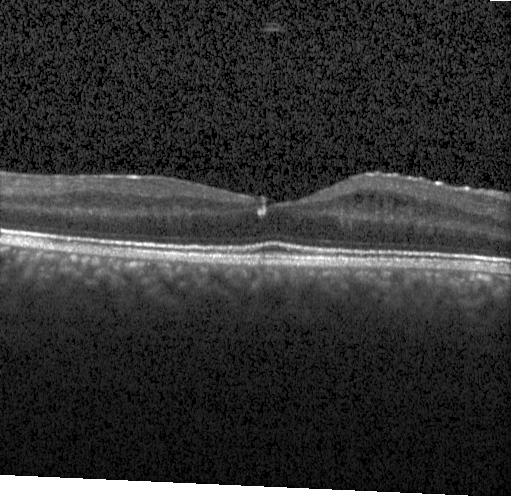

Diabetic macular edema (DME).